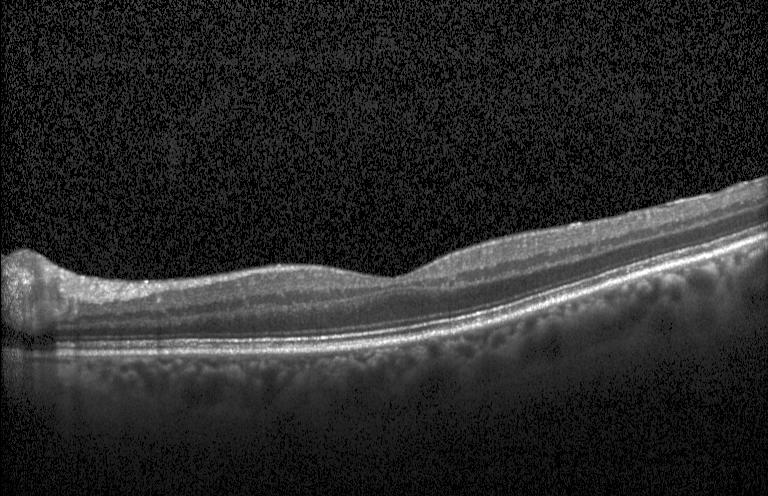 Retinal OCT B-scan. Instrument: Heidelberg Spectralis. Spectral-domain optical coherence tomography.
Neither choroidal neovascularization, diabetic macular edema, nor drusen.